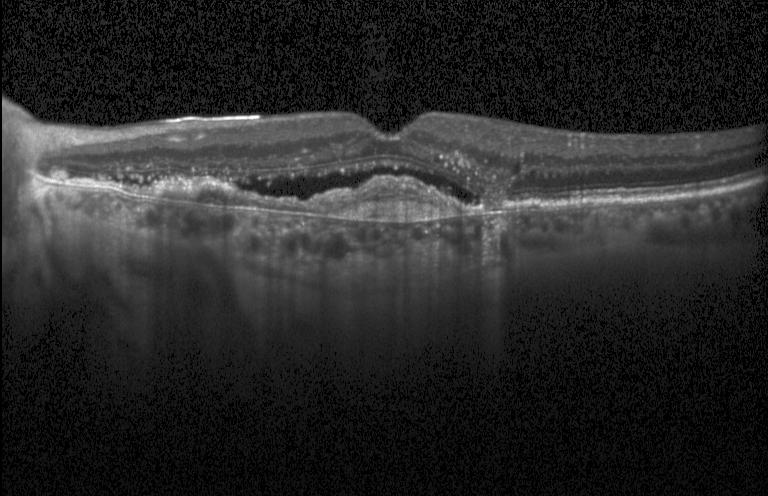
Acquired on a Heidelberg Spectralis, optical coherence tomography scan, spectral-domain OCT.
Diagnosis: a choroidal neovascular membrane.